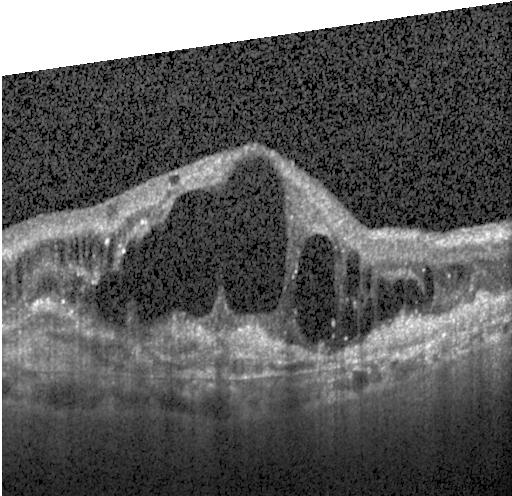
Dx: CNV.